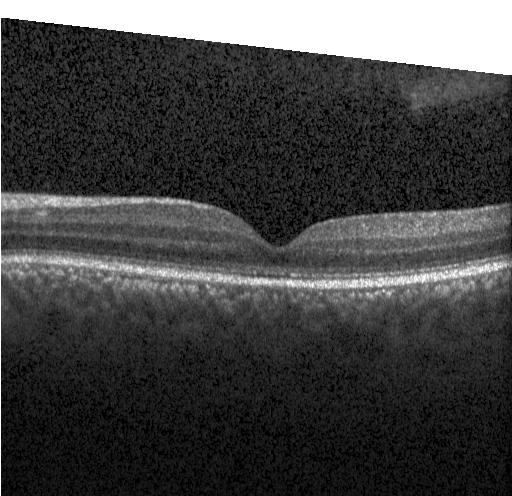

No CNV, DME, or drusen.